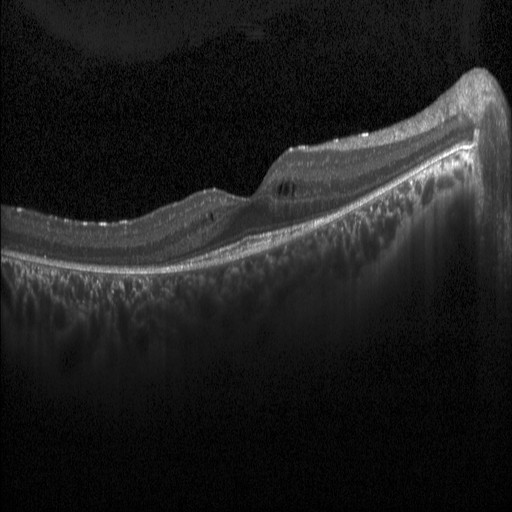

Retinal OCT cross-section.
Dx: diabetic macular edema.